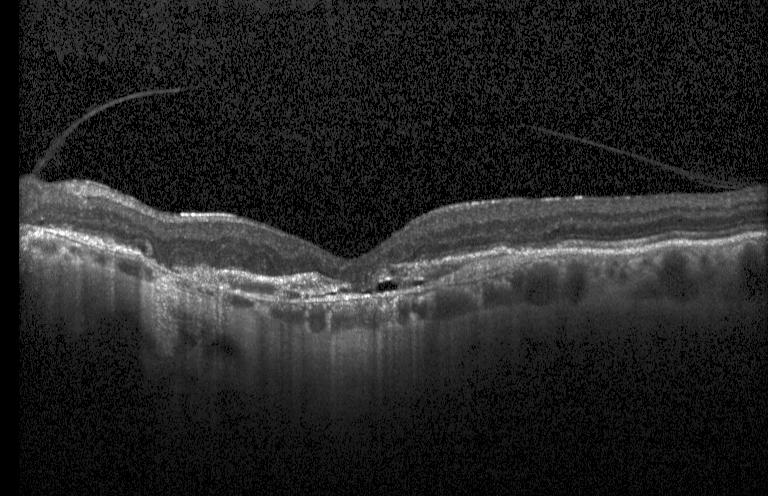
Horizontal scan through the fovea, Heidelberg Spectralis OCT system, spectral-domain OCT, OCT line scan. Choroidal neovascularization.